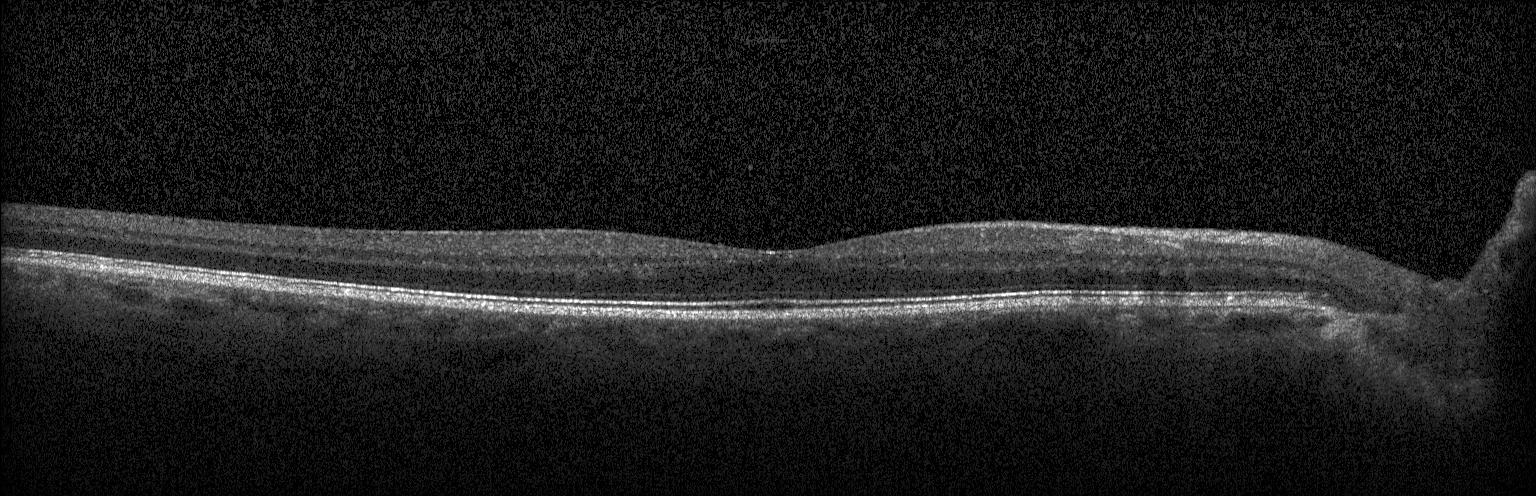 Retinal OCT cross-section, through the macula.
Macular OCT: no evidence of choroidal neovascularization, diabetic macular edema, or drusen.